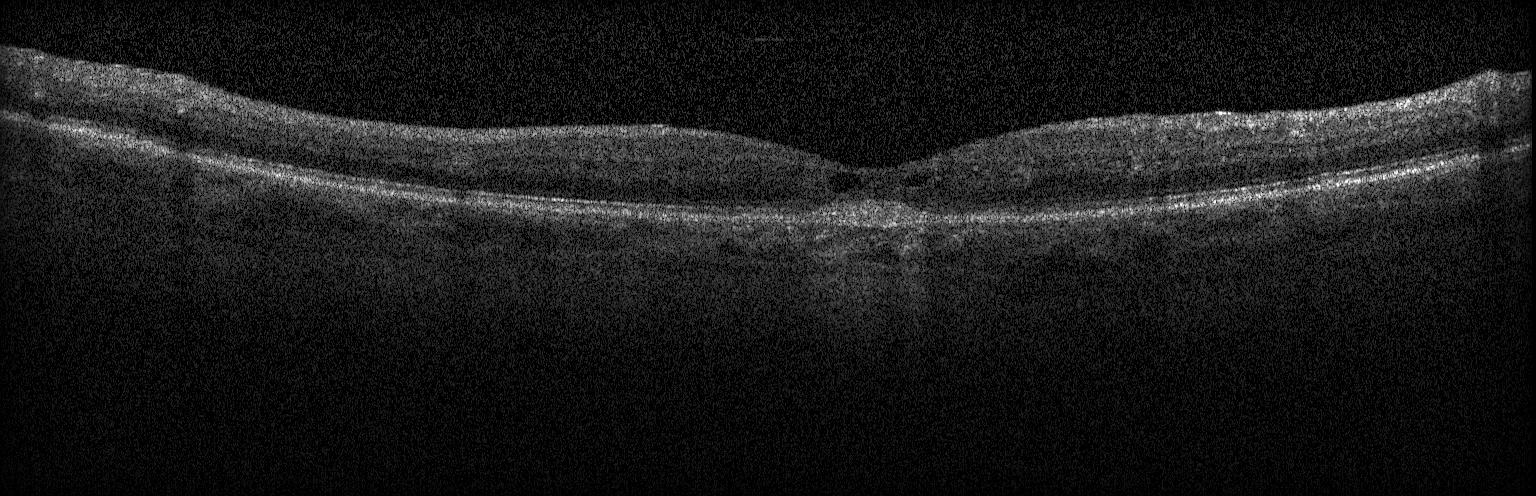
Finding: choroidal neovascularization.